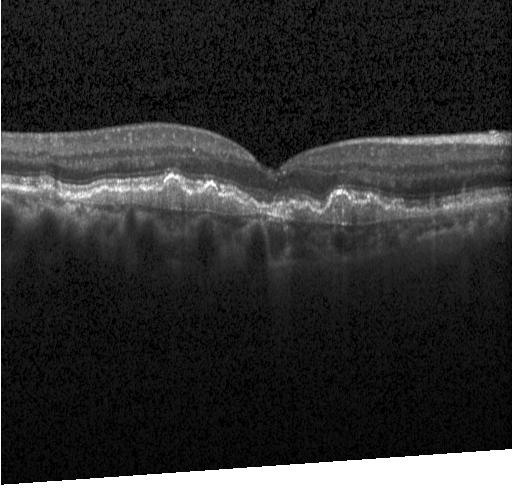 OCT B-scan · spectral-domain optical coherence tomography · Heidelberg Spectralis.
Impression: CNV.